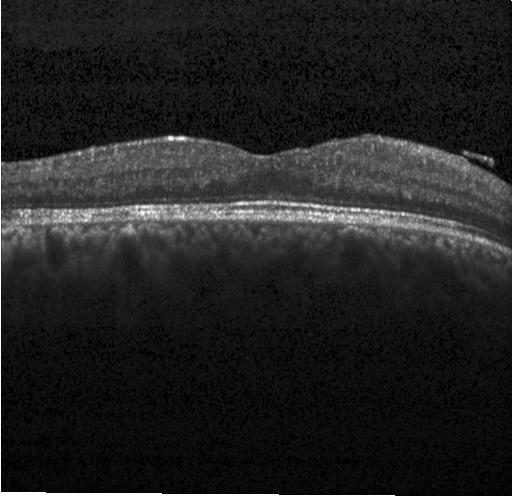

Retinal OCT cross-section; Heidelberg Spectralis; macular scan
OCT finding: no evidence of CNV, DME, or drusen.